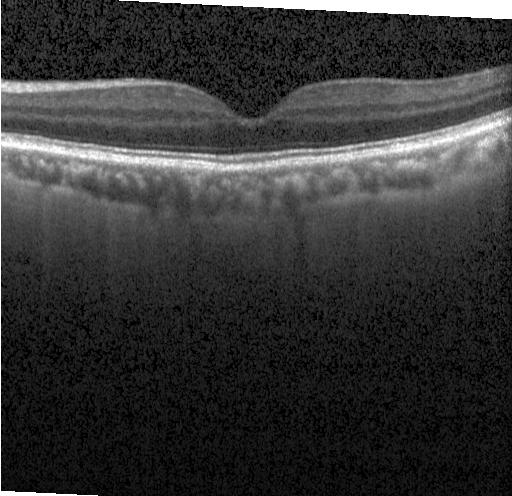

OCT scan showing neither CNV, DME, nor drusen.